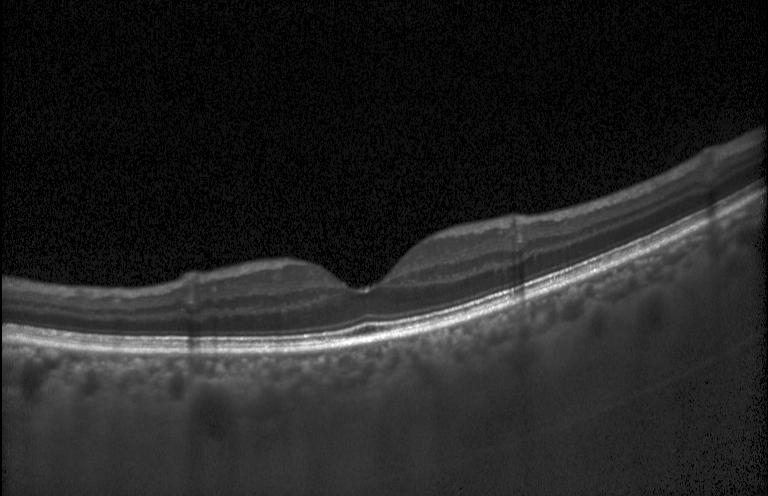 Spectral-domain OCT B-scan: no CNV, no DME, and no drusen.